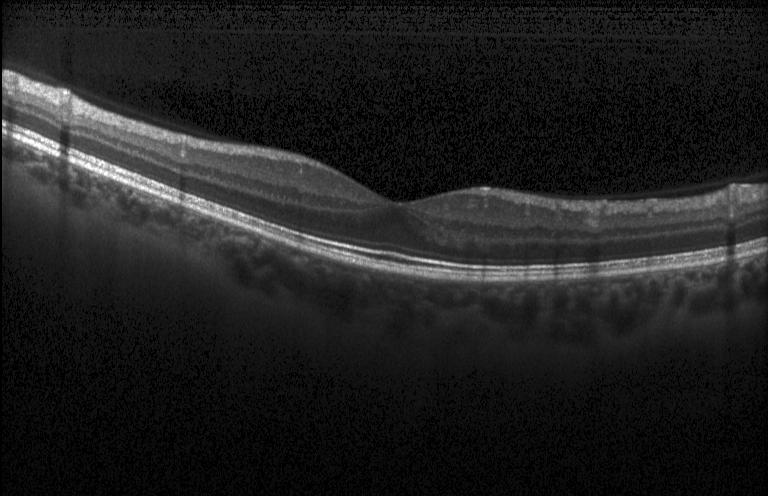 Macular OCT: neither CNV, DME, nor drusen.